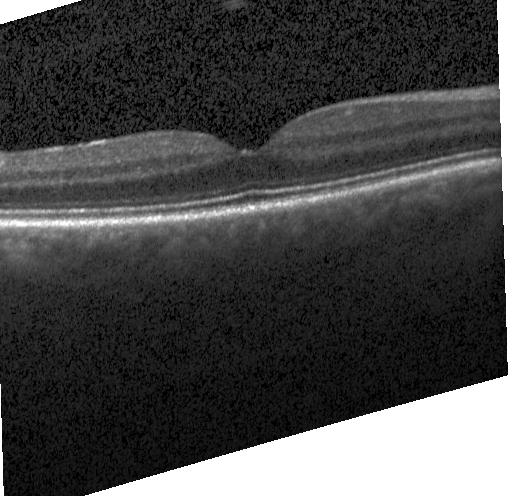
Retinal OCT cross-section, Heidelberg Spectralis, macular scan, spectral-domain optical coherence tomography. Assessment: no CNV, no DME, and no drusen.